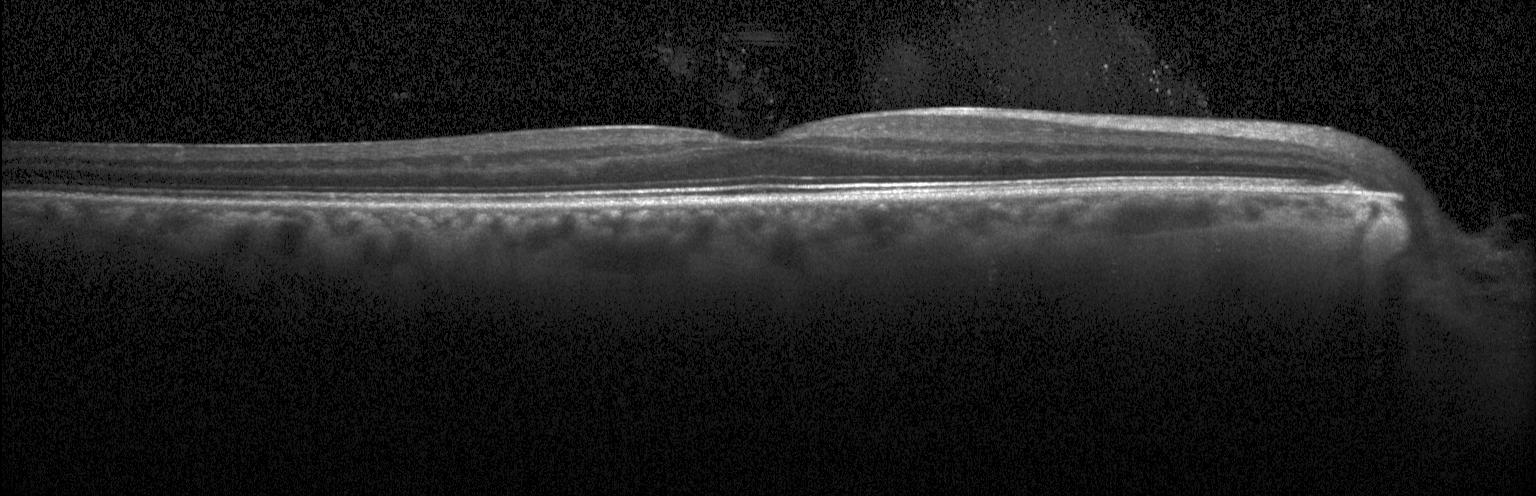 OCT B-scan. Macular OCT: no evidence of CNV, DME, or drusen.